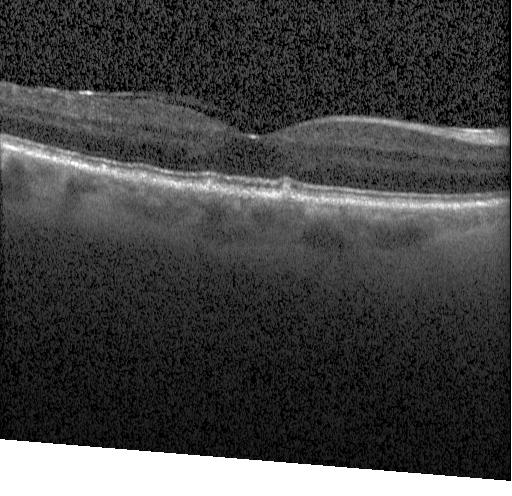

Diagnosis: sub-RPE drusenoid deposits.